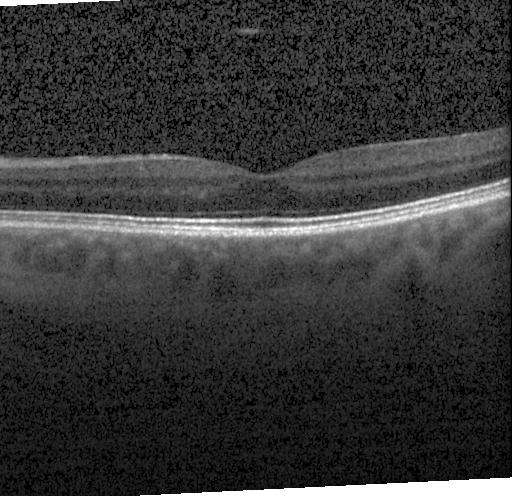

Spectral-domain optical coherence tomography; retinal OCT cross-section. Diagnosis: no evidence of choroidal neovascularization, diabetic macular edema, or drusen.